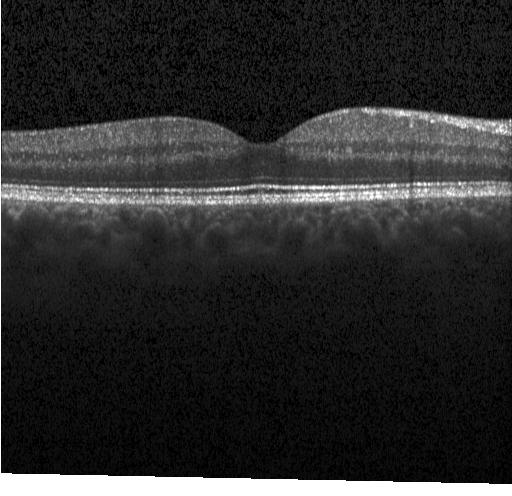

Diagnosis: no evidence of choroidal neovascularization, diabetic macular edema, or drusen.